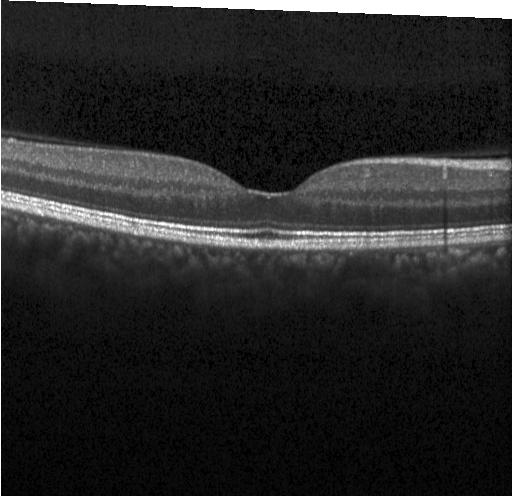 Spectral-domain optical coherence tomography; optical coherence tomography scan.
Impression: neither CNV, DME, nor drusen.